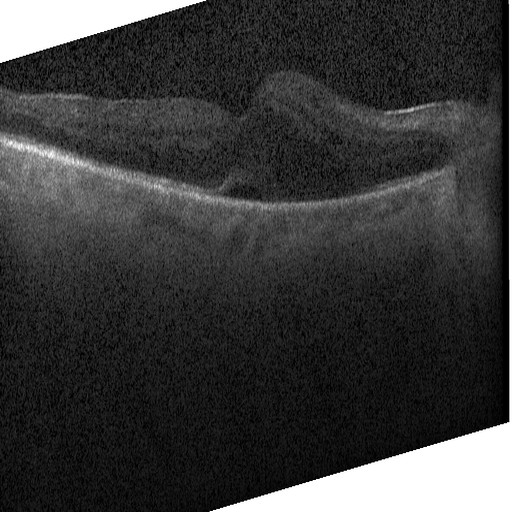

Spectral-domain optical coherence tomography; centered on the fovea; OCT B-scan — The scan shows diabetic macular edema (DME).